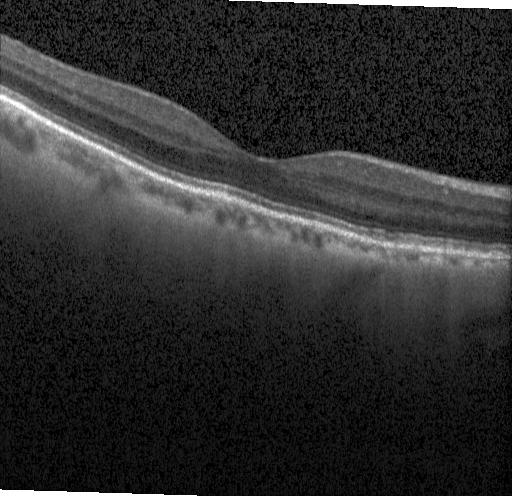 Finding: no CNV, no DME, and no drusen.